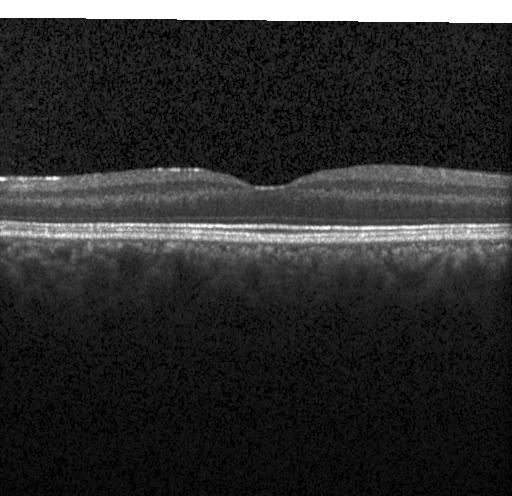
Optical coherence tomography scan · Heidelberg Spectralis OCT system.
Finding: no evidence of choroidal neovascularization, diabetic macular edema, or drusen.